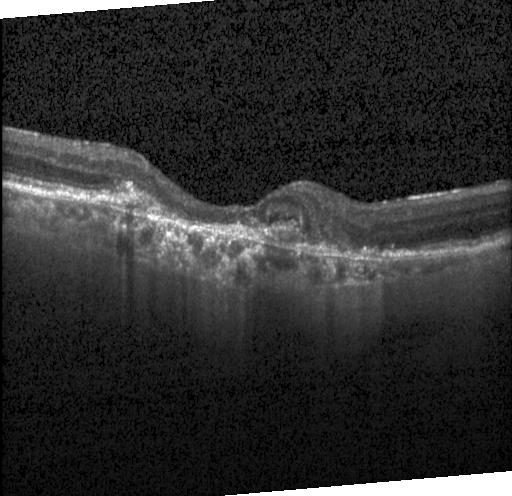
Dx: a choroidal neovascular membrane.